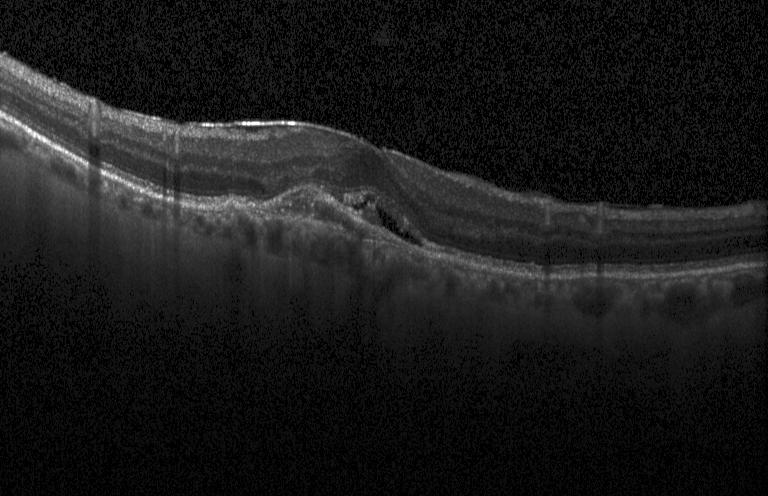 Choroidal neovascularization (CNV).